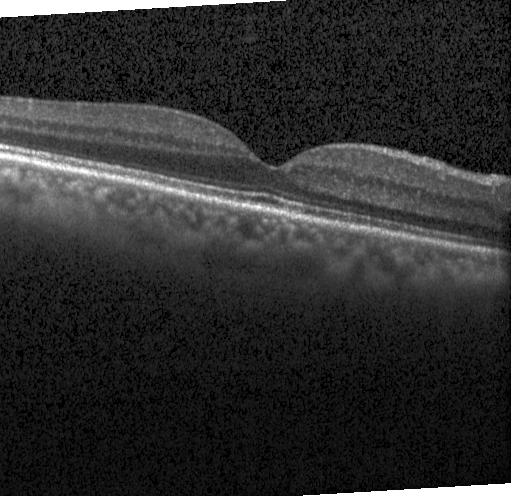
OCT line scan. Instrument: Heidelberg Spectralis. Horizontal scan through the fovea.
Dx: no CNV, no DME, and no drusen.